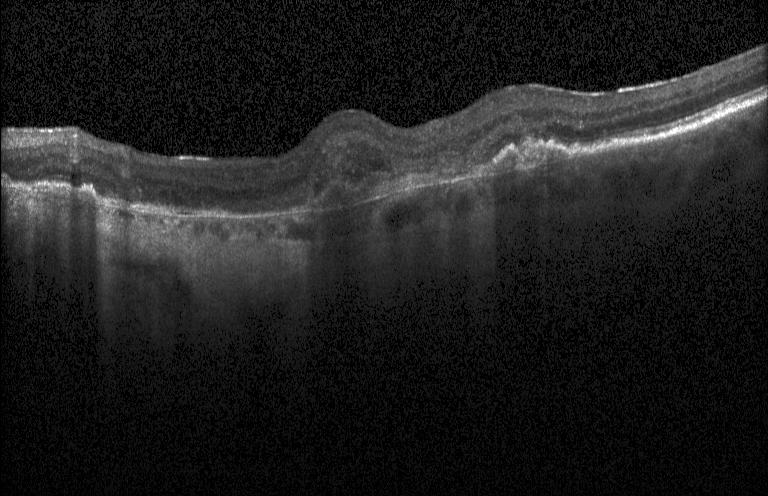 Heidelberg Spectralis OCT system. SD-OCT. Optical coherence tomography B-scan — This B-scan demonstrates choroidal neovascularization (CNV).